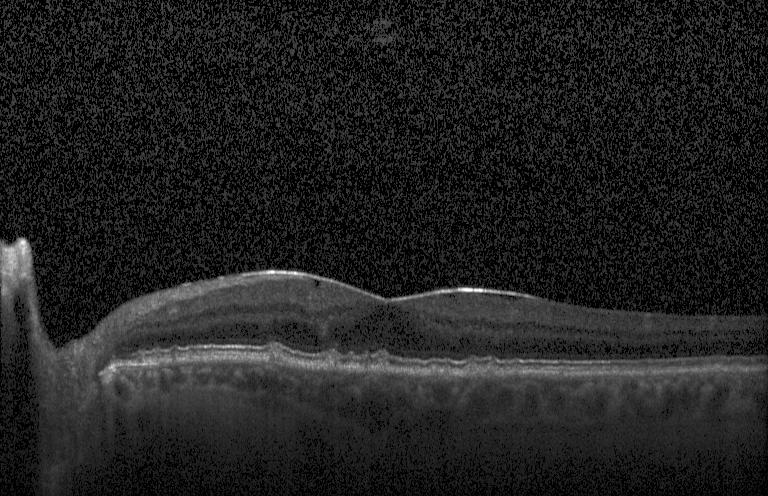

Finding: drusen.